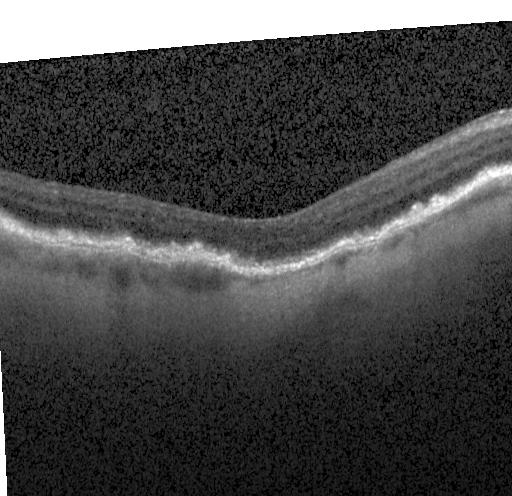 Spectral-domain optical coherence tomography. OCT line scan. Horizontal scan through the fovea. OCT finding: a choroidal neovascular membrane.